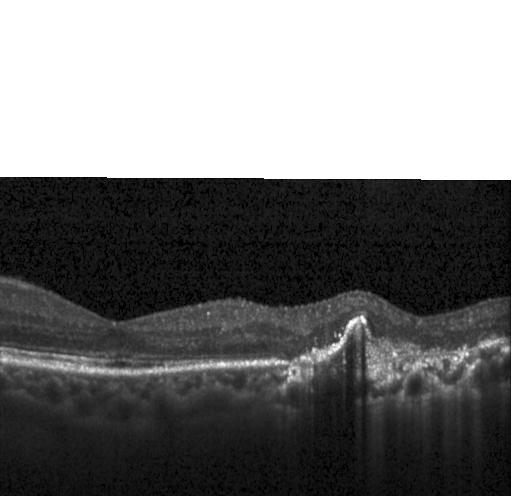 Macular OCT demonstrating a choroidal neovascular membrane.